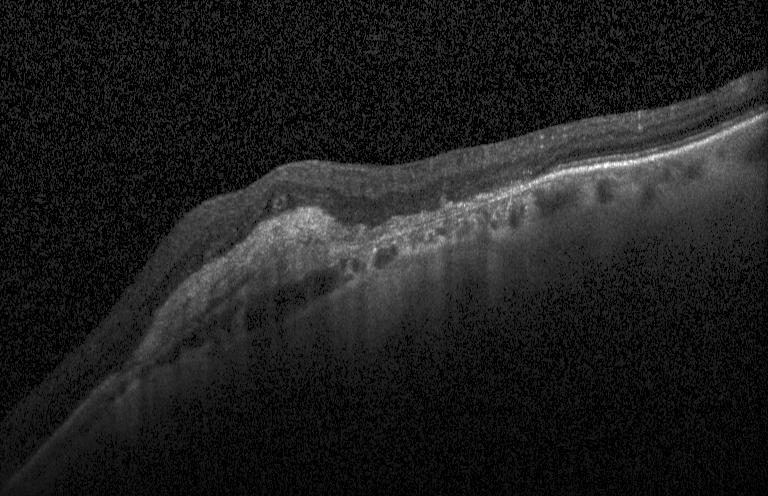
Horizontal scan through the fovea. Retinal OCT cross-section. Heidelberg Spectralis OCT system
A choroidal neovascular membrane.